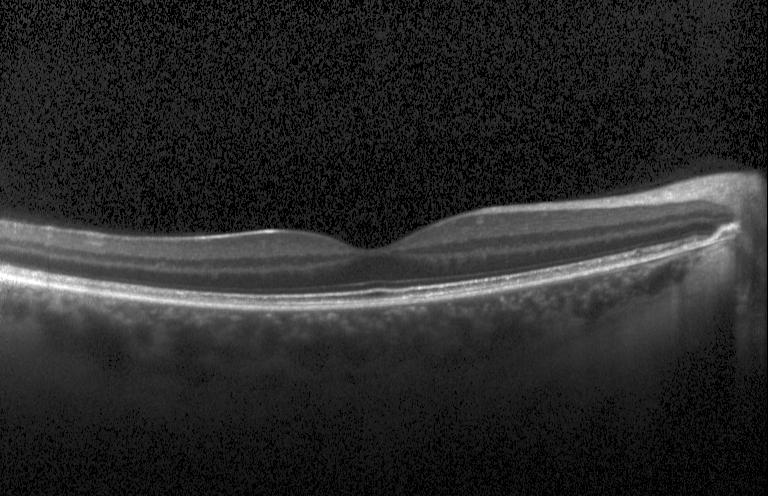
Instrument: Heidelberg Spectralis. Retinal OCT B-scan. Spectral-domain optical coherence tomography. Centered on the fovea.
Finding: no choroidal neovascularization, diabetic macular edema, or drusen.